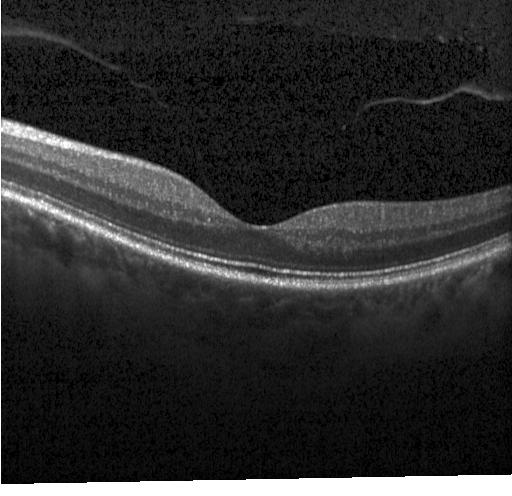

Assessment: neither CNV, DME, nor drusen.